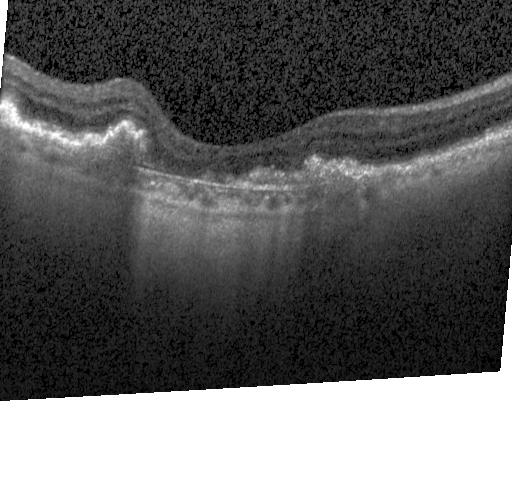

OCT line scan; through the macula; SD-OCT. OCT finding: choroidal neovascularization (CNV).